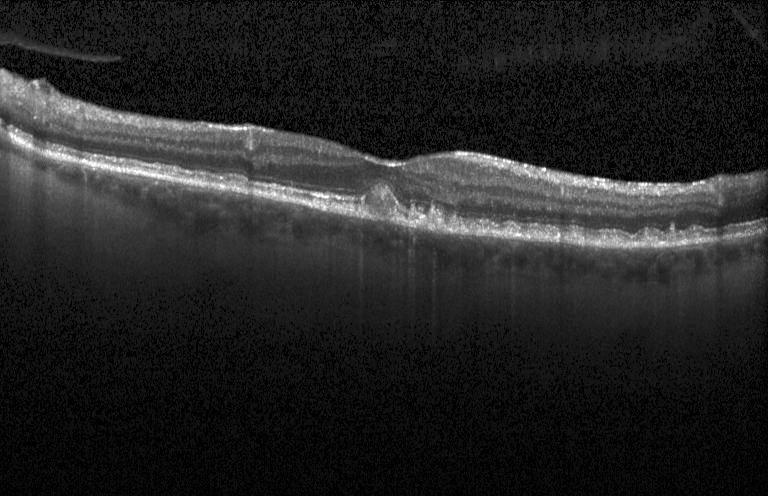 Optical coherence tomography B-scan · Heidelberg Spectralis · horizontal scan through the fovea.
Macular OCT: multiple drusen.